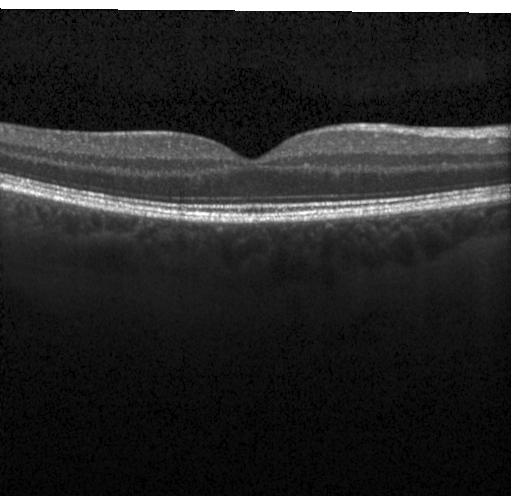
OCT line scan. Spectral-domain optical coherence tomography. Through the macula. Heidelberg Spectralis — Impression: neither choroidal neovascularization, diabetic macular edema, nor drusen.